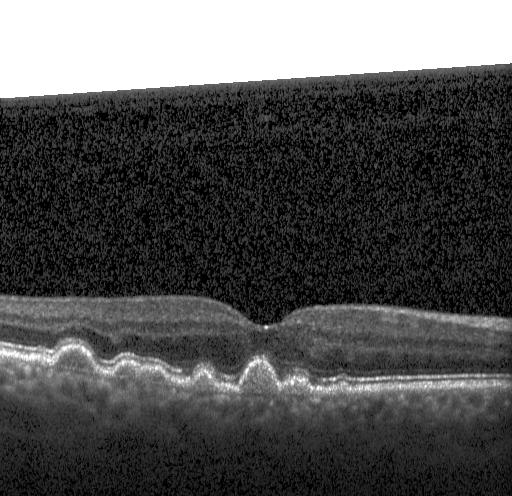 Optical coherence tomography B-scan.
Diagnosis: multiple drusen.